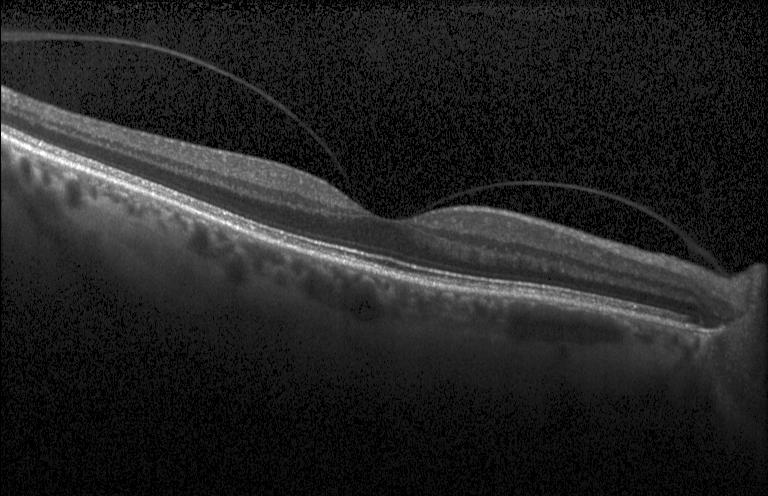
OCT B-scan. Finding: no evidence of choroidal neovascularization, diabetic macular edema, or drusen.